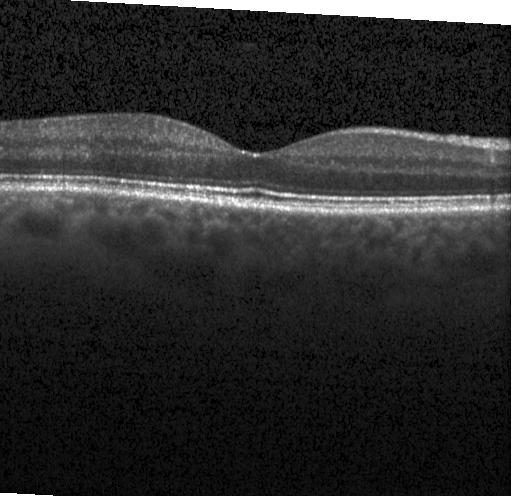 SD-OCT, retinal OCT B-scan — Diagnosis: no evidence of CNV, DME, or drusen.